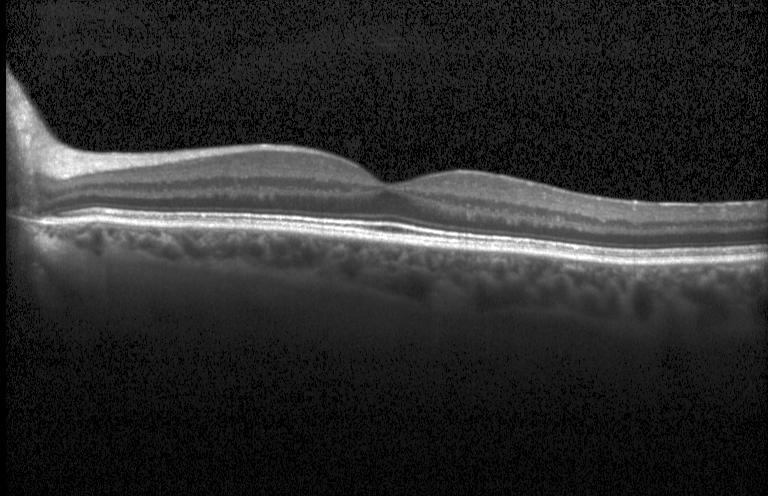 Macular OCT: no choroidal neovascularization, no diabetic macular edema, and no drusen.